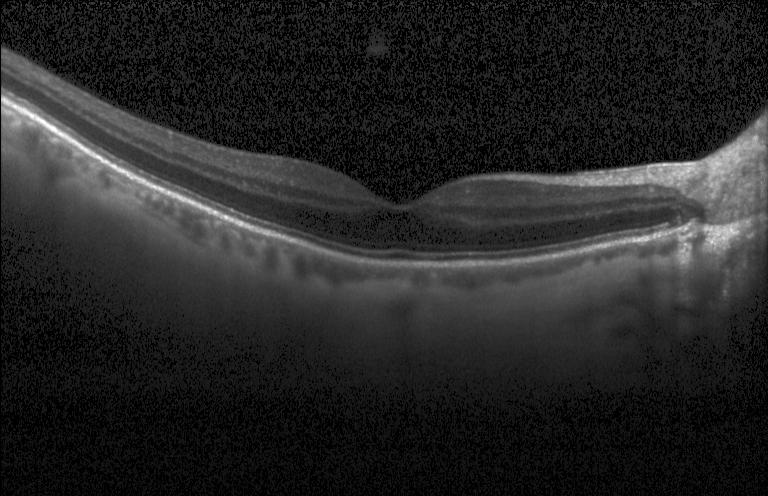 No choroidal neovascularization, no diabetic macular edema, and no drusen.